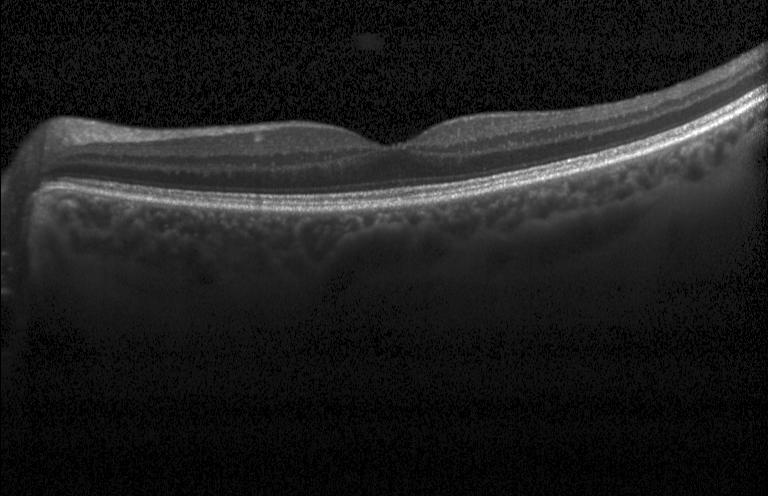
Dx: neither choroidal neovascularization, diabetic macular edema, nor drusen.